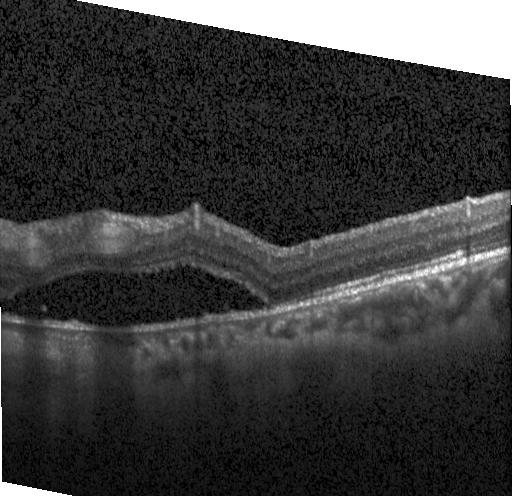

Retinal OCT cross-section showing a choroidal neovascular membrane.